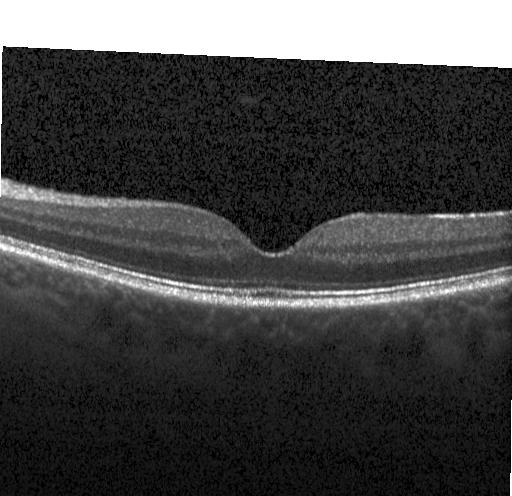 Spectral-domain optical coherence tomography, macular scan, Heidelberg Spectralis, retinal OCT B-scan
Diagnosis: no choroidal neovascularization, diabetic macular edema, or drusen.